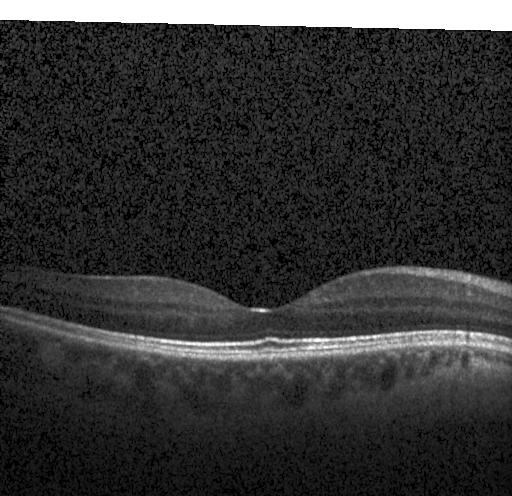 OCT finding: no choroidal neovascularization, diabetic macular edema, or drusen.